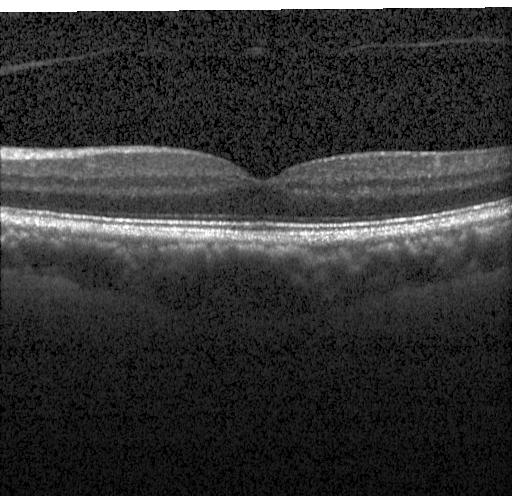 Optical coherence tomography scan · macular scan · instrument: Heidelberg Spectralis · SD-OCT. Finding: no CNV, DME, or drusen.